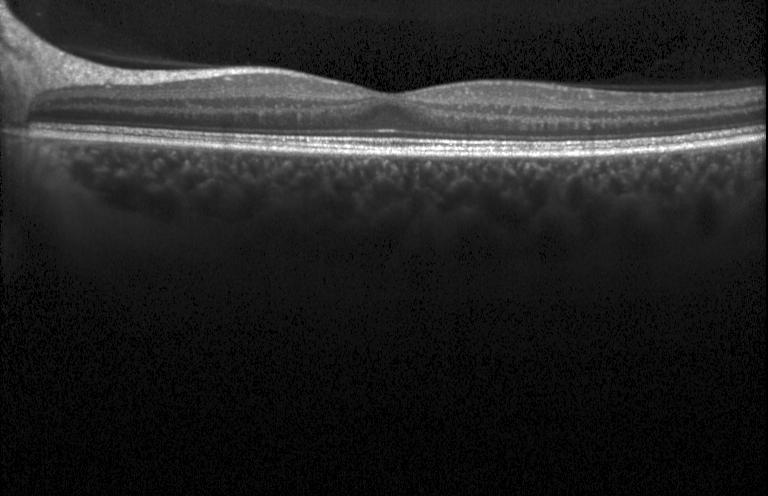 Retinal OCT cross-section. Heidelberg Spectralis. Horizontal scan through the fovea. Spectral-domain optical coherence tomography — This B-scan demonstrates no choroidal neovascularization, diabetic macular edema, or drusen.